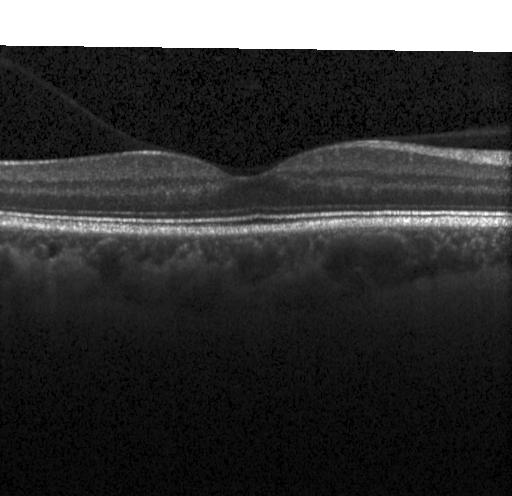
SD-OCT. Horizontal scan through the fovea. Heidelberg Spectralis OCT system. OCT B-scan — No evidence of choroidal neovascularization, diabetic macular edema, or drusen.